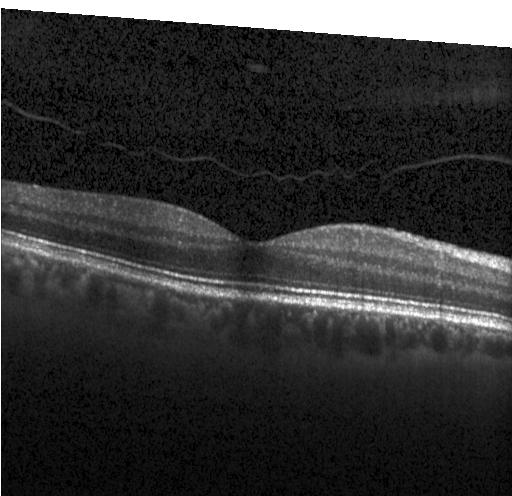
Spectral-domain OCT B-scan: no CNV, no DME, and no drusen.